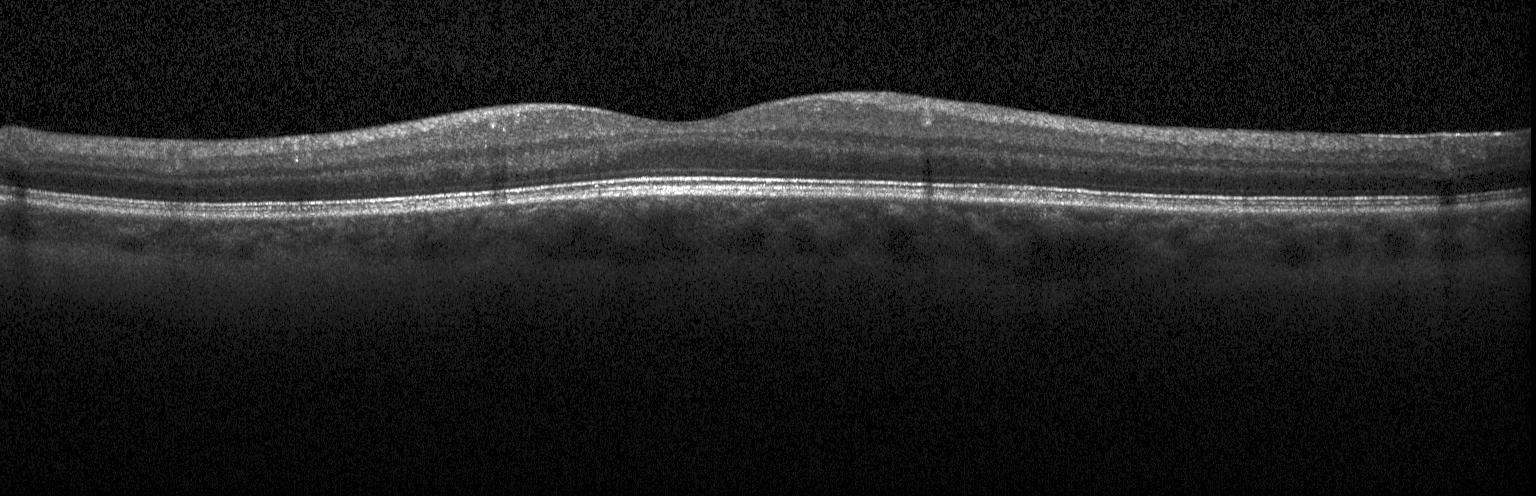

Optical coherence tomography B-scan, SD-OCT, acquired on a Heidelberg Spectralis, macular scan — Macular OCT: neither choroidal neovascularization, diabetic macular edema, nor drusen.